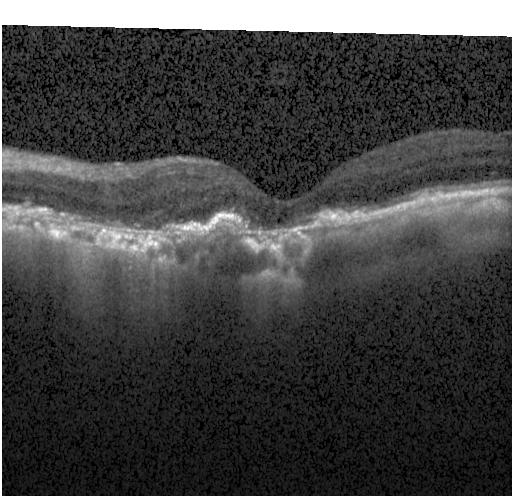

Instrument: Heidelberg Spectralis · optical coherence tomography scan — Finding: a choroidal neovascular membrane.